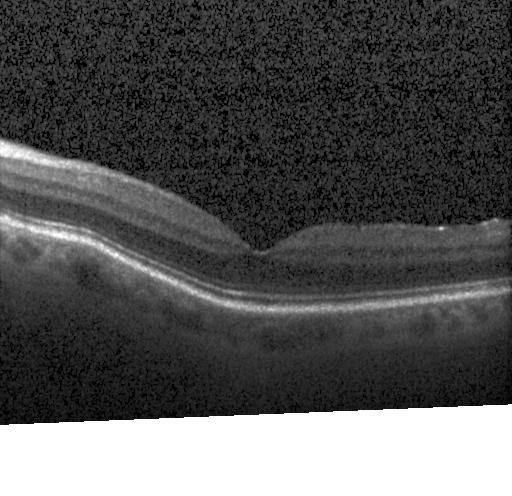 Instrument: Heidelberg Spectralis · SD-OCT · optical coherence tomography B-scan. The scan shows neither CNV, DME, nor drusen.